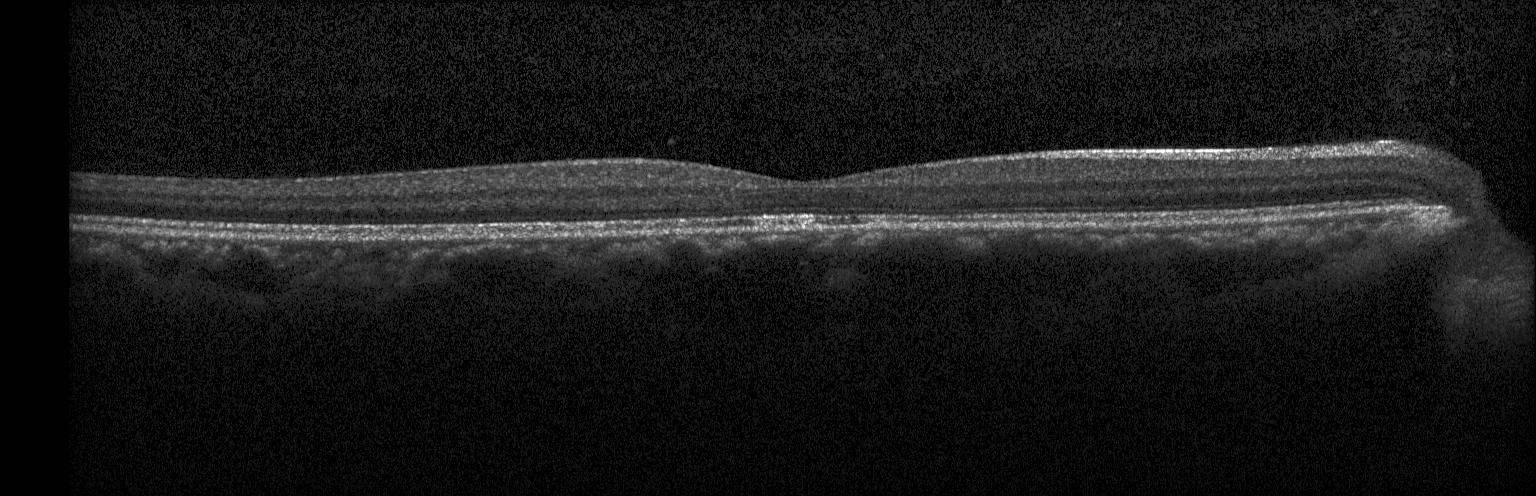 OCT B-scan, horizontal scan through the fovea, Heidelberg Spectralis OCT system.
Impression: no CNV, DME, or drusen.